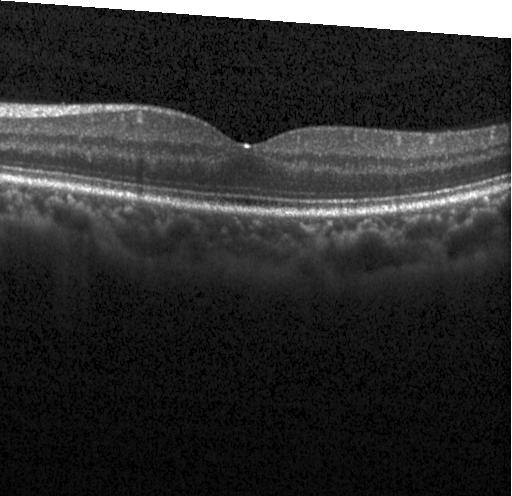 Fovea-centered; retinal OCT B-scan
The scan shows no CNV, no DME, and no drusen.